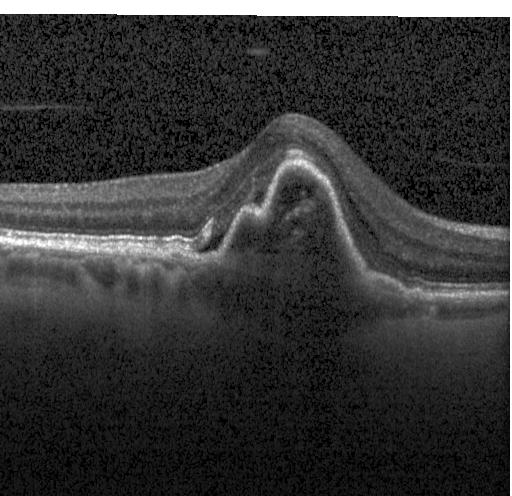

Retinal OCT cross-section.
Impression: a choroidal neovascular membrane.